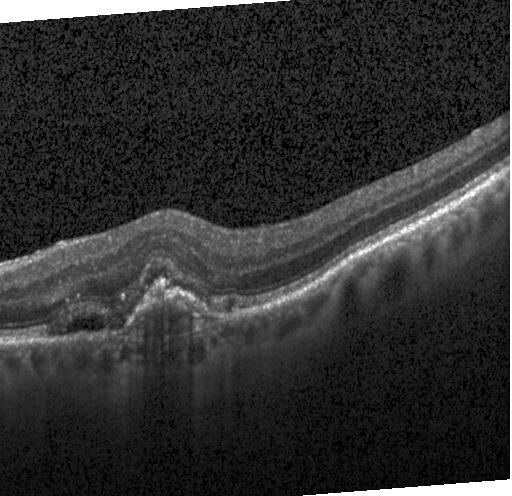

Macular OCT: CNV.